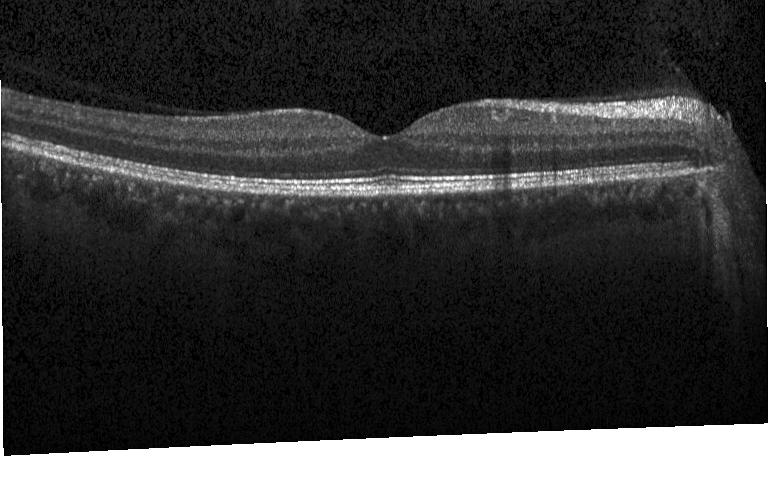

OCT line scan.
Impression: neither choroidal neovascularization, diabetic macular edema, nor drusen.